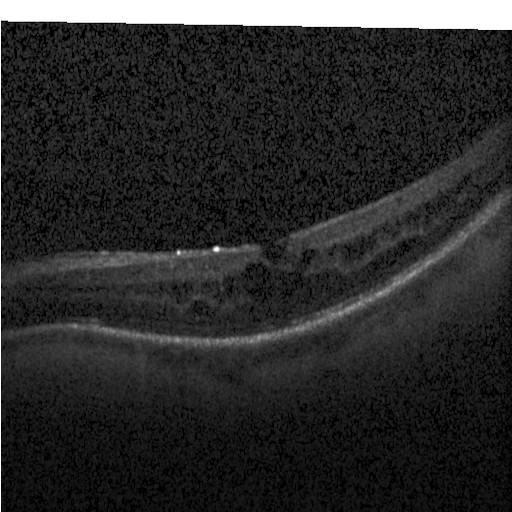 OCT finding: diabetic macular edema (DME).